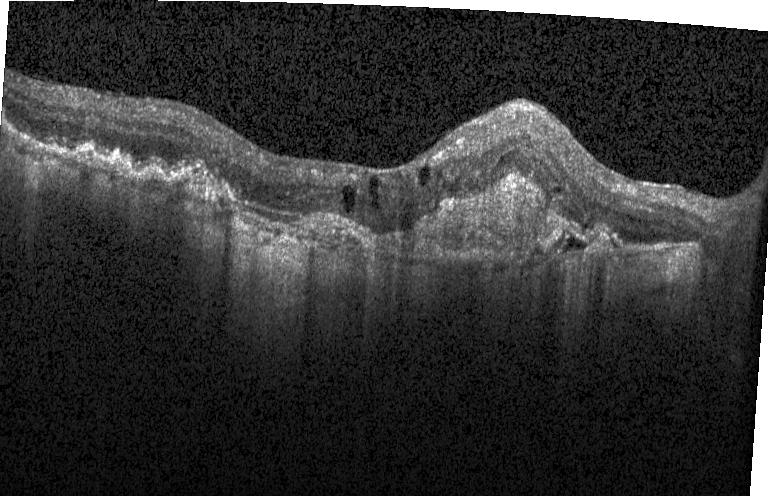

Diagnosis: CNV.